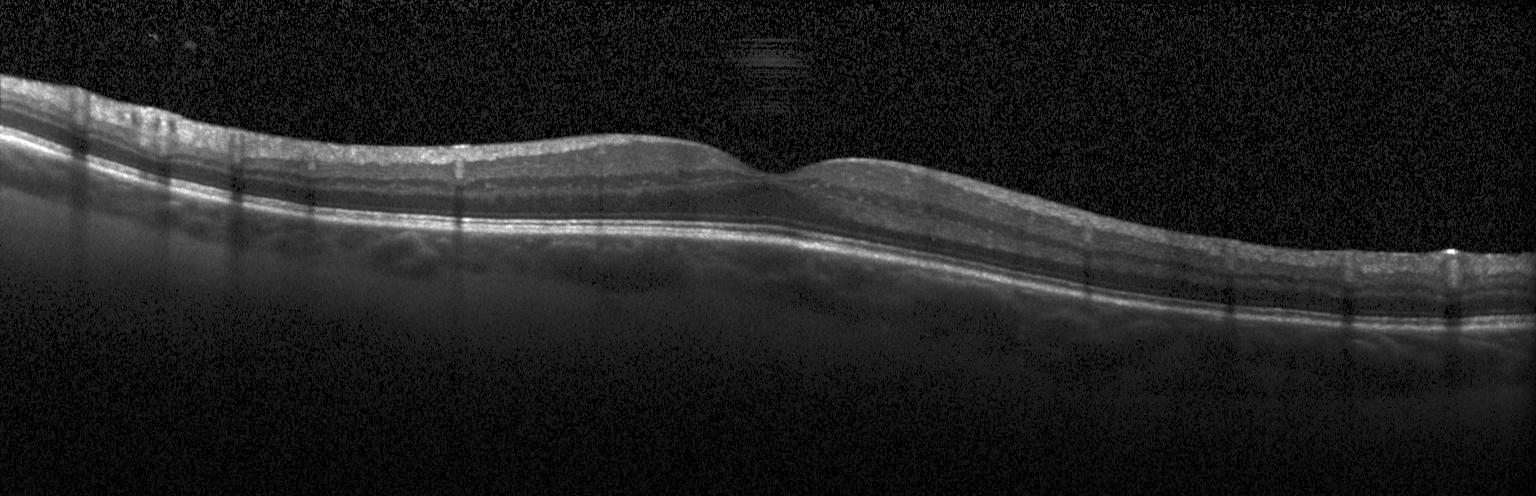 Diagnosis: no choroidal neovascularization, diabetic macular edema, or drusen.